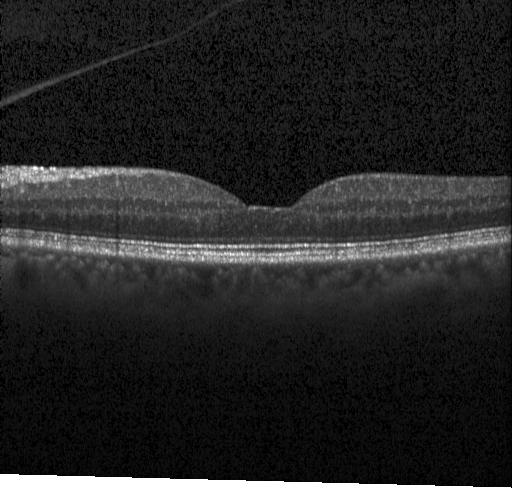

Heidelberg Spectralis. Horizontal scan through the fovea. OCT B-scan
Impression: no evidence of choroidal neovascularization, diabetic macular edema, or drusen.